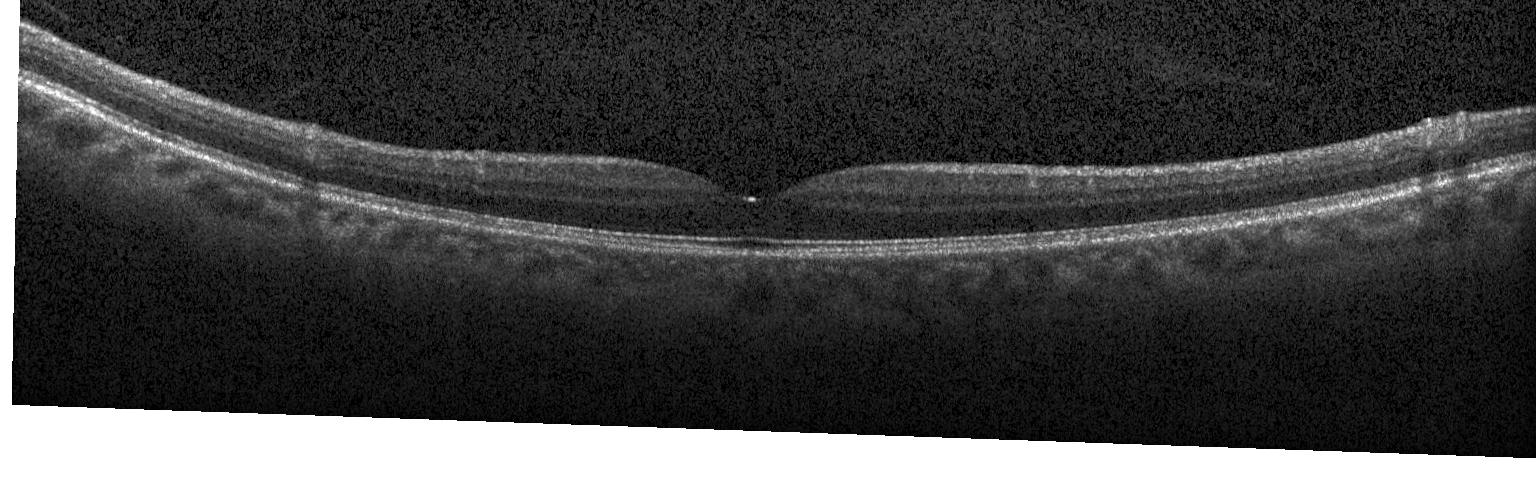

Impression: neither choroidal neovascularization, diabetic macular edema, nor drusen.